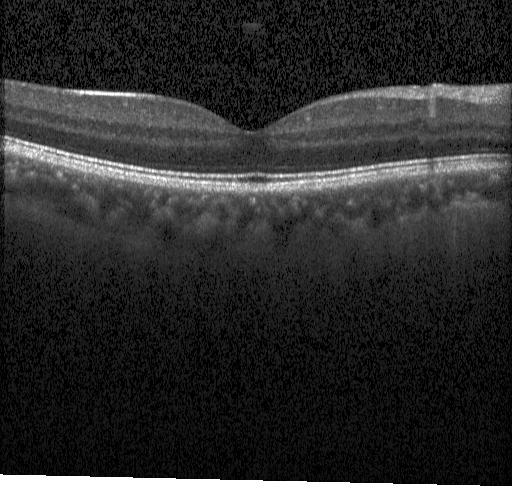
Assessment: neither CNV, DME, nor drusen.